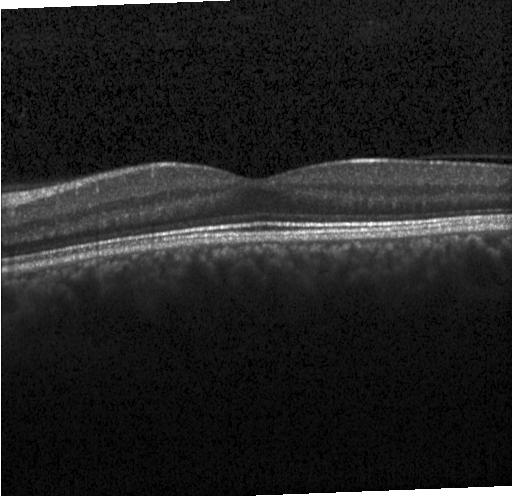
Through the macula · spectral-domain OCT · Heidelberg Spectralis · OCT line scan
Diagnosis: neither CNV, DME, nor drusen.